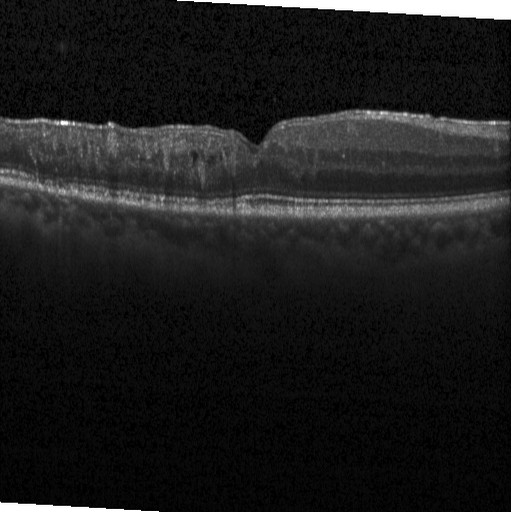 Retinal OCT cross-section showing DME.